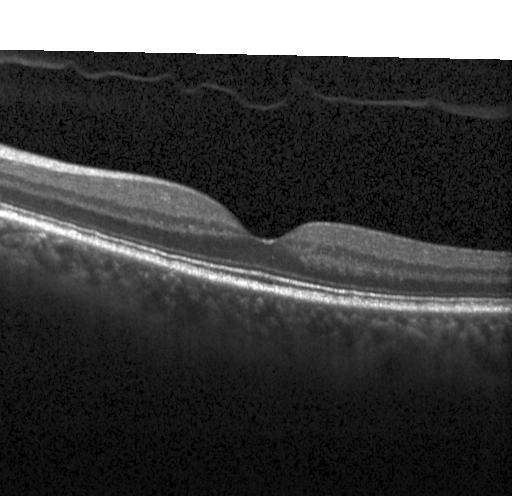

Finding: neither CNV, DME, nor drusen.